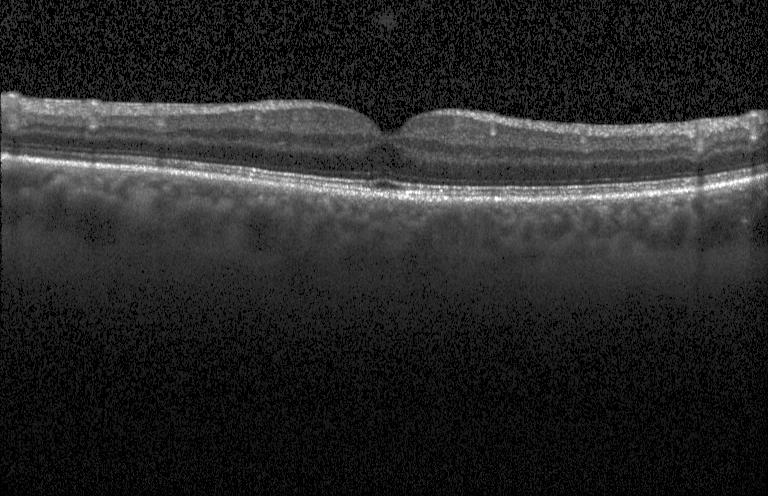

Diagnosis: no evidence of CNV, DME, or drusen.